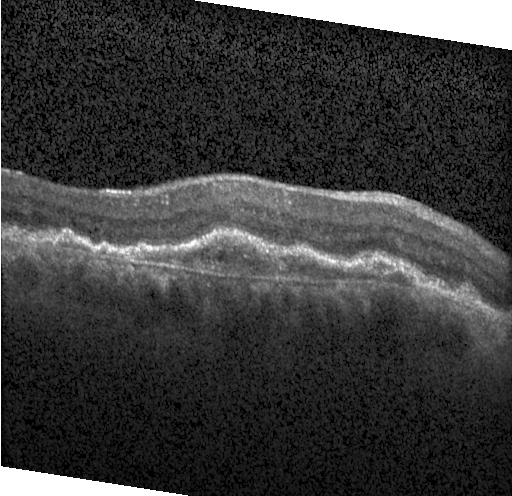

Retinal OCT cross-section showing choroidal neovascularization (CNV).